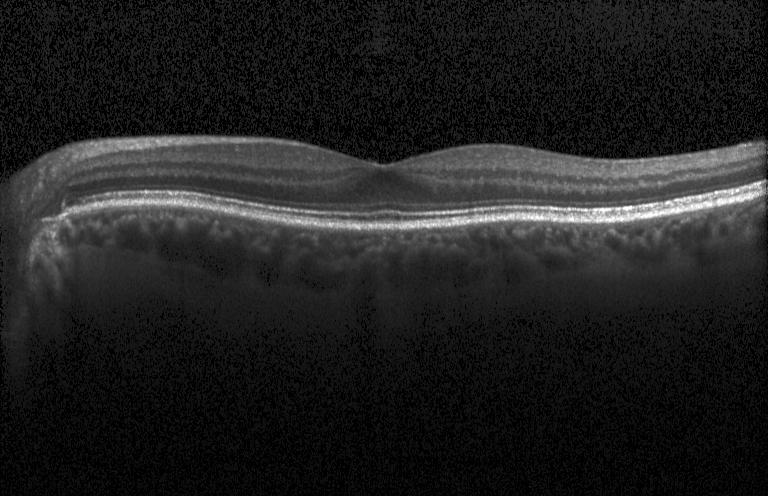

Acquired on a Heidelberg Spectralis, OCT line scan — The scan shows no evidence of choroidal neovascularization, diabetic macular edema, or drusen.